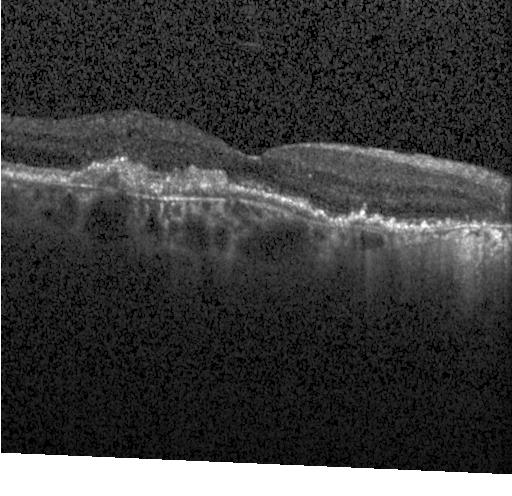

Through the macula · optical coherence tomography B-scan.
Choroidal neovascularization (CNV).